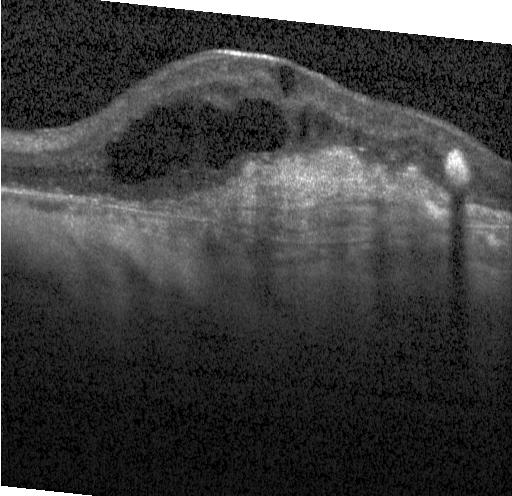 Retinal OCT cross-section showing CNV.